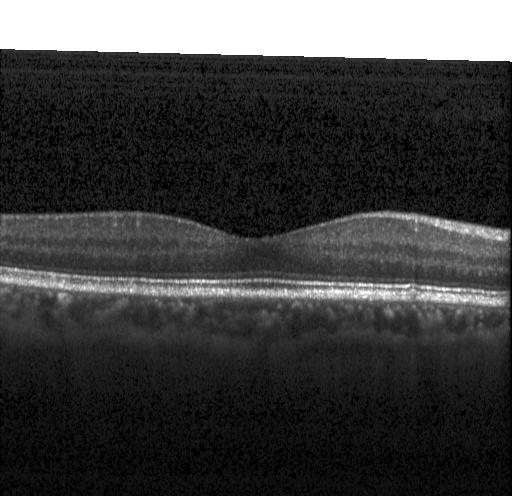 Spectral-domain optical coherence tomography; centered on the fovea; Heidelberg Spectralis; retinal OCT B-scan.
OCT finding: no CNV, DME, or drusen.